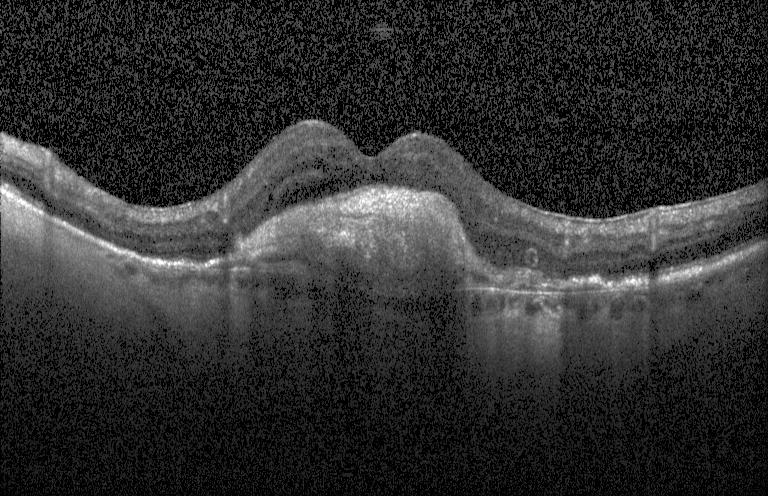
Finding: a choroidal neovascular membrane.